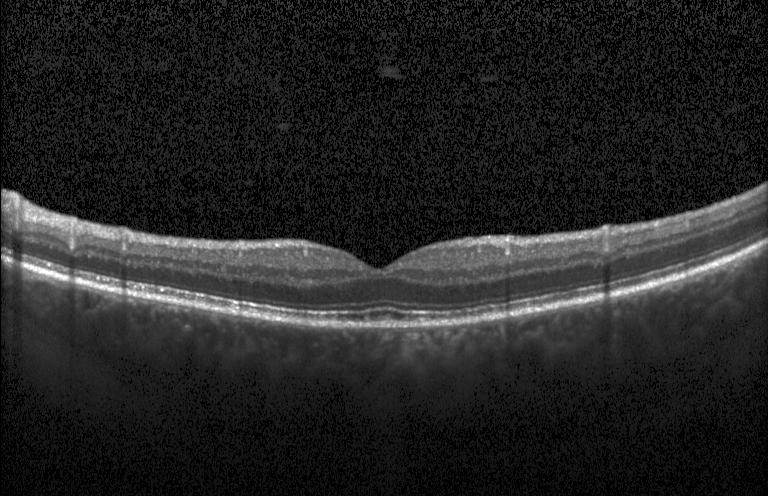

Heidelberg Spectralis · OCT B-scan.
Macular OCT: no CNV, DME, or drusen.